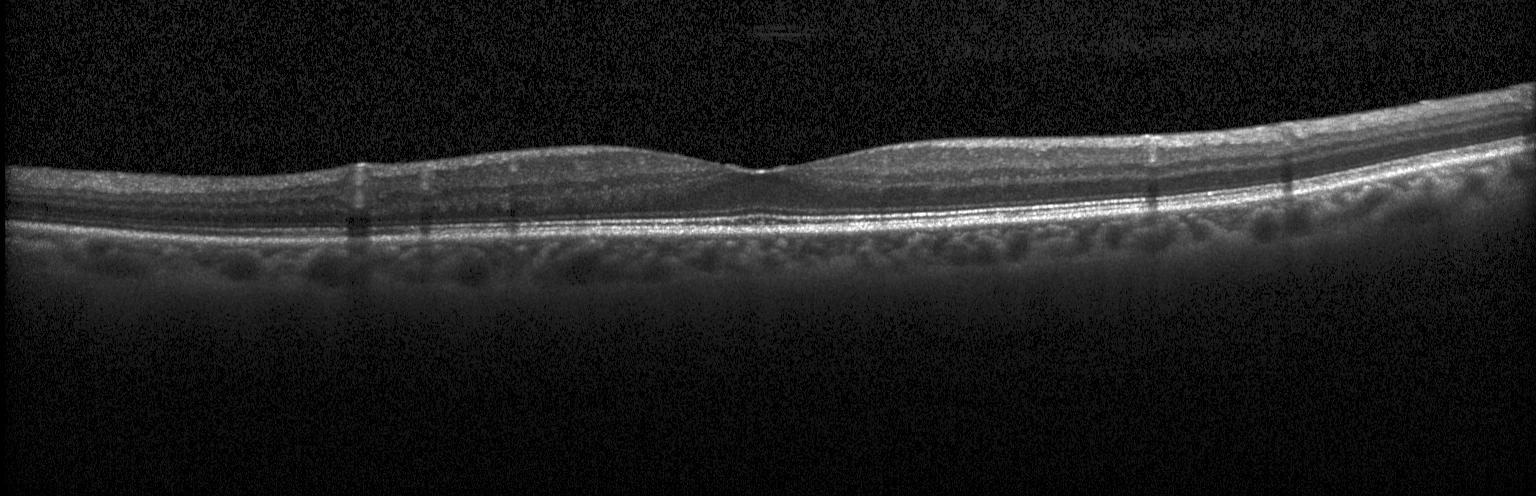

Diagnosis: no choroidal neovascularization, no diabetic macular edema, and no drusen.